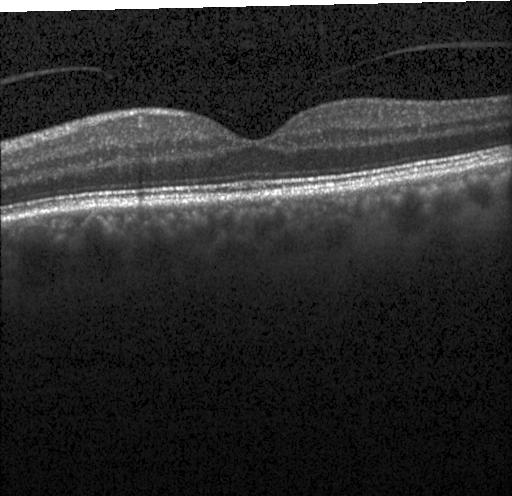
Diagnosis: no CNV, DME, or drusen.